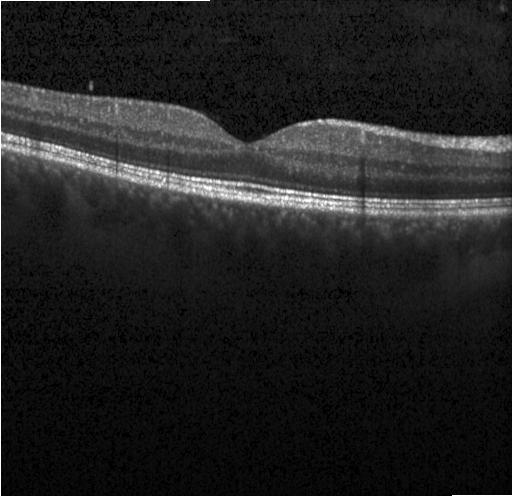
Optical coherence tomography B-scan — Diagnosis: neither choroidal neovascularization, diabetic macular edema, nor drusen.